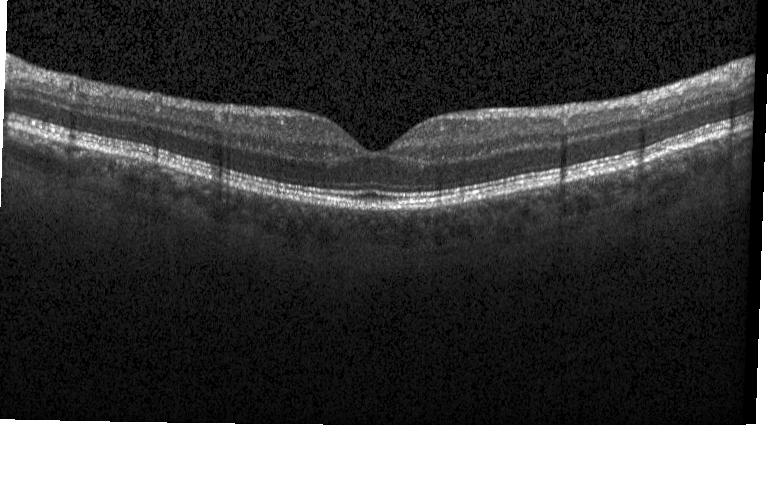 No choroidal neovascularization, no diabetic macular edema, and no drusen.